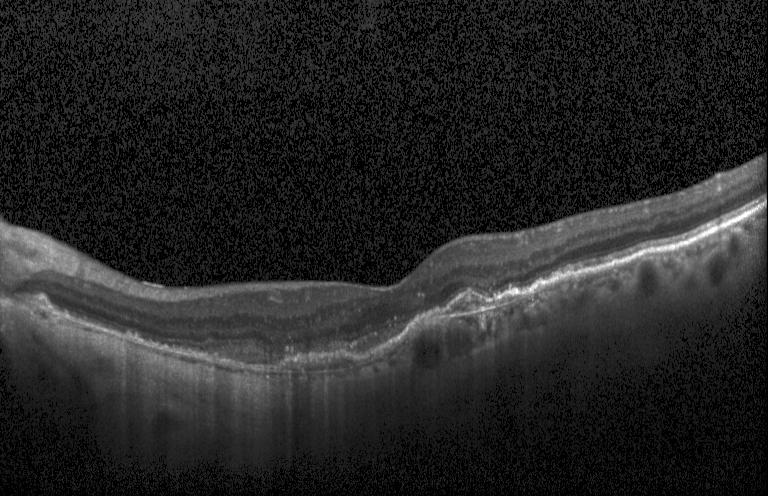
Acquired on a Heidelberg Spectralis · optical coherence tomography B-scan.
Diagnosis: choroidal neovascularization (CNV).